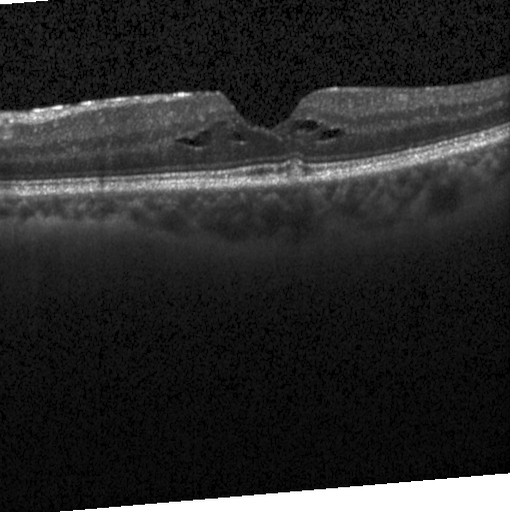
Retinal OCT B-scan
The scan shows diabetic macular edema (DME).